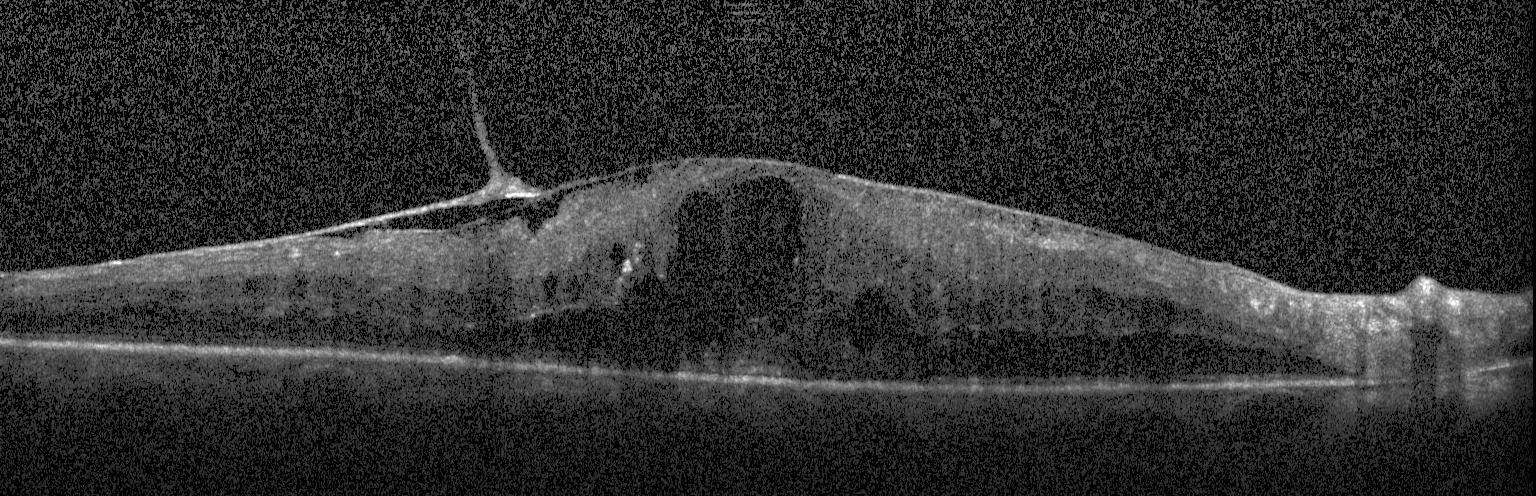

Macular OCT demonstrating diabetic macular edema.